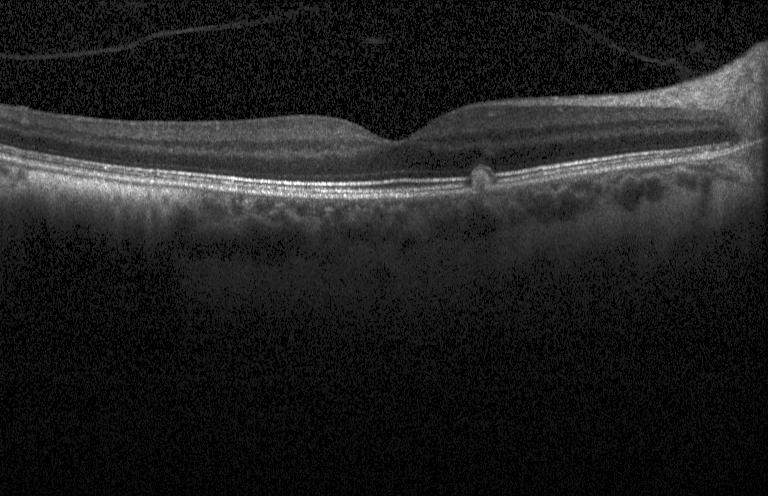
Diagnosis: drusen.